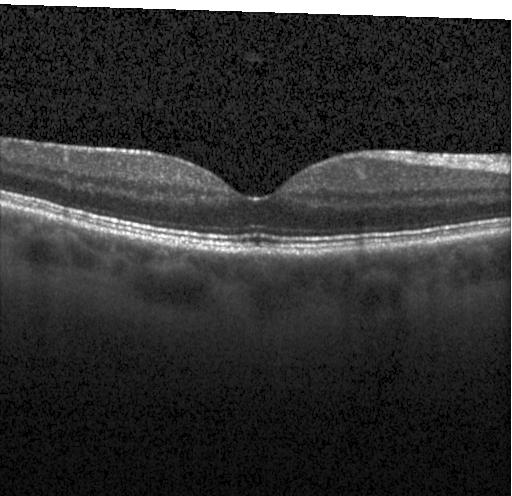
SD-OCT; OCT B-scan; instrument: Heidelberg Spectralis — Assessment: no choroidal neovascularization, no diabetic macular edema, and no drusen.